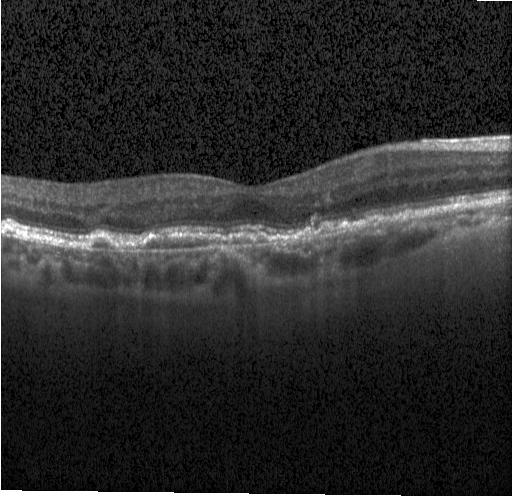
Optical coherence tomography scan
Finding: a choroidal neovascular membrane.